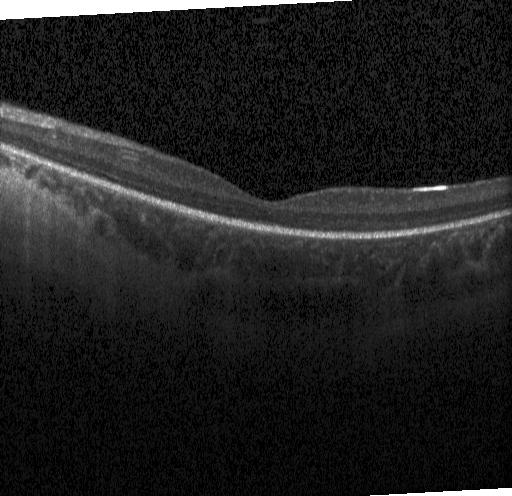
Spectral-domain OCT, centered on the fovea, Heidelberg Spectralis OCT system, retinal OCT cross-section. Dx: no choroidal neovascularization, diabetic macular edema, or drusen.